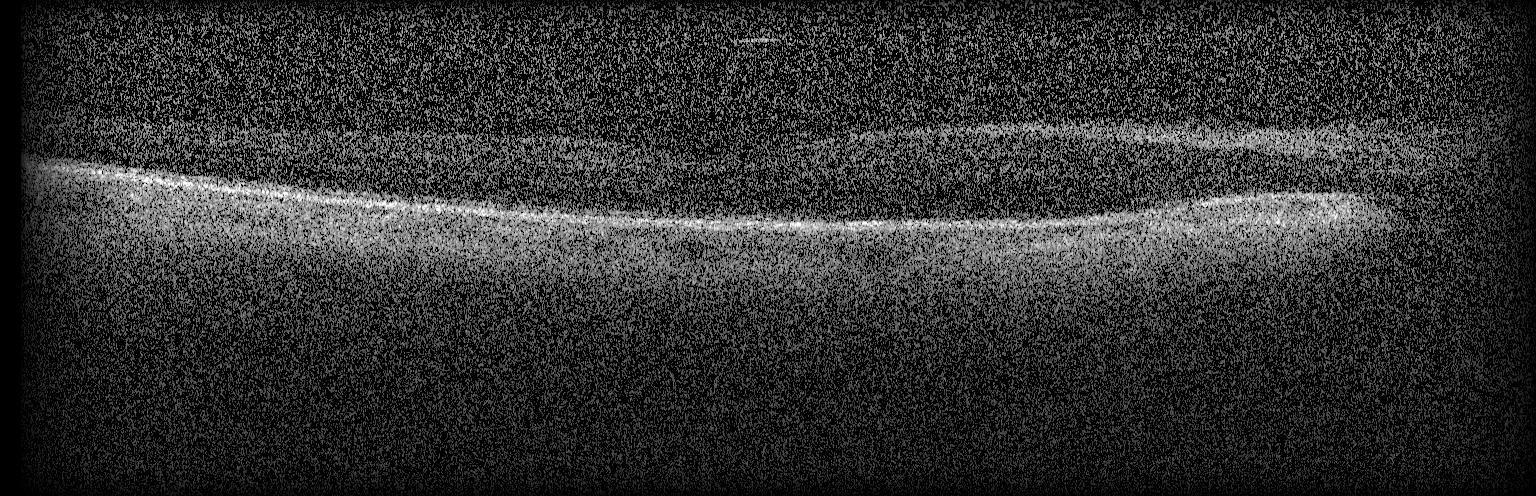
Retinal OCT cross-section, Heidelberg Spectralis, macular scan, spectral-domain OCT. Finding: no CNV, no DME, and no drusen.